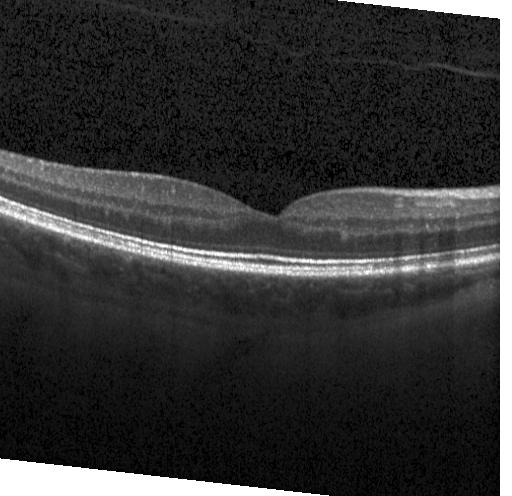 Optical coherence tomography scan — The scan shows no choroidal neovascularization, no diabetic macular edema, and no drusen.